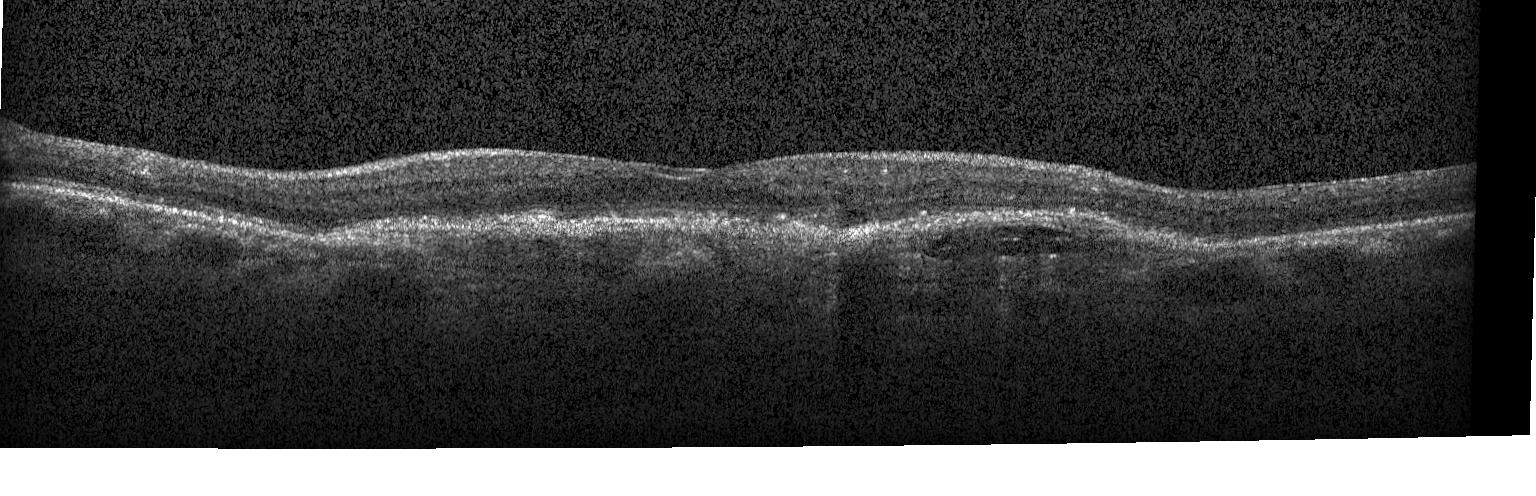
Retinal OCT B-scan, centered on the fovea. The scan shows a choroidal neovascular membrane.